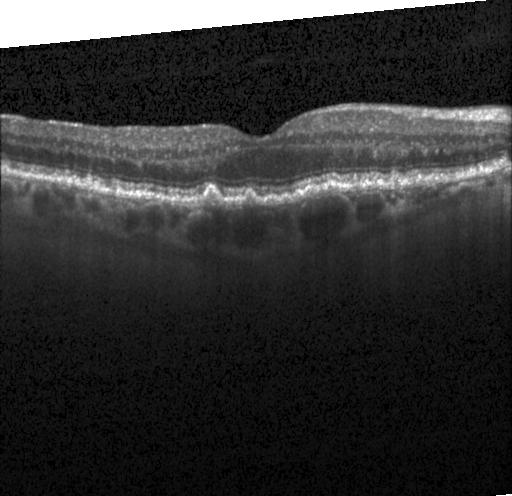
Centered on the fovea. OCT line scan. Diagnosis: drusen.